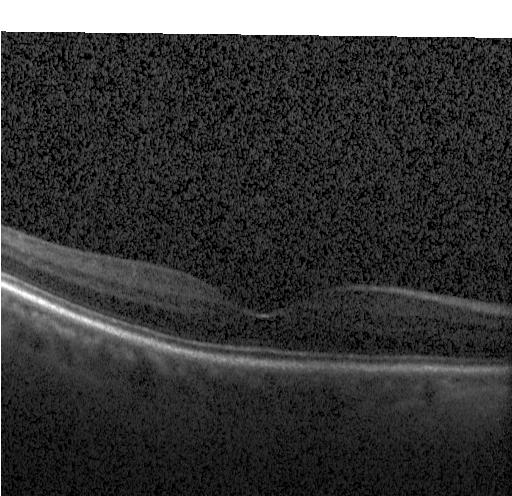
Spectral-domain OCT B-scan: no choroidal neovascularization, no diabetic macular edema, and no drusen.